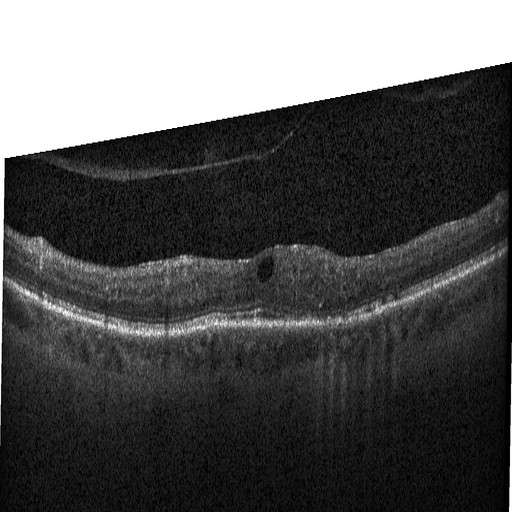 Fovea-centered, SD-OCT, OCT line scan, instrument: Heidelberg Spectralis
OCT finding: DME.